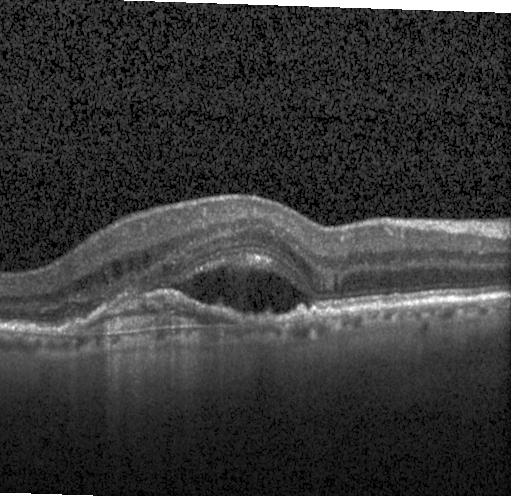 Diagnosis: a choroidal neovascular membrane.